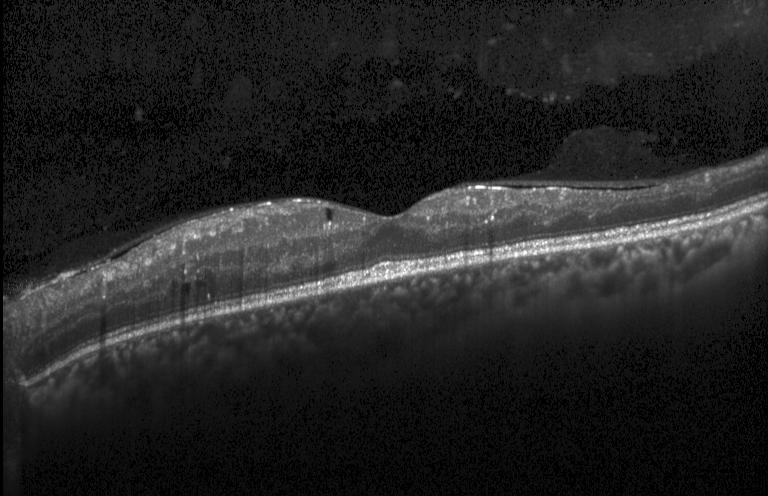

Retinal OCT cross-section showing diabetic macular edema.